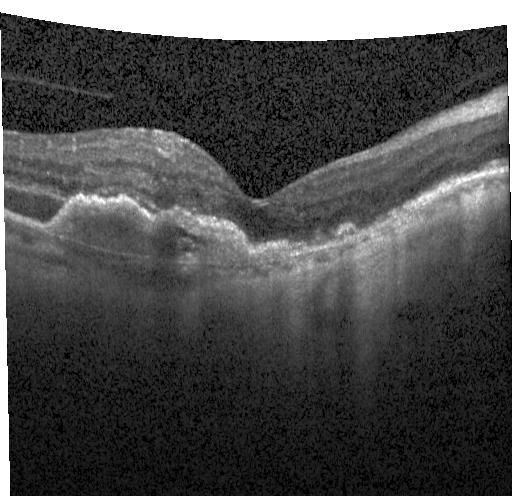 Retinal OCT cross-section. Spectral-domain optical coherence tomography
Macular OCT: a choroidal neovascular membrane.